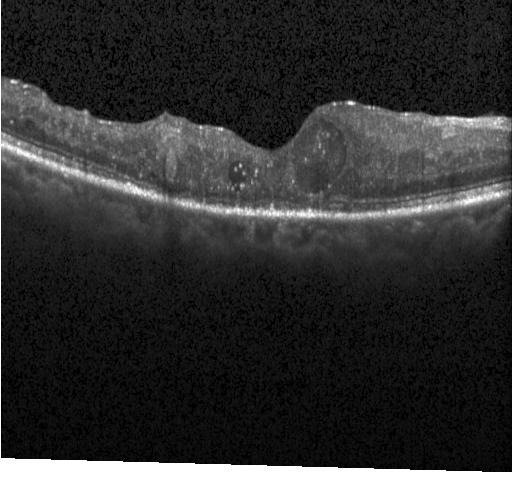 OCT B-scan · Heidelberg Spectralis OCT system · macular scan.
Diagnosis: DME.